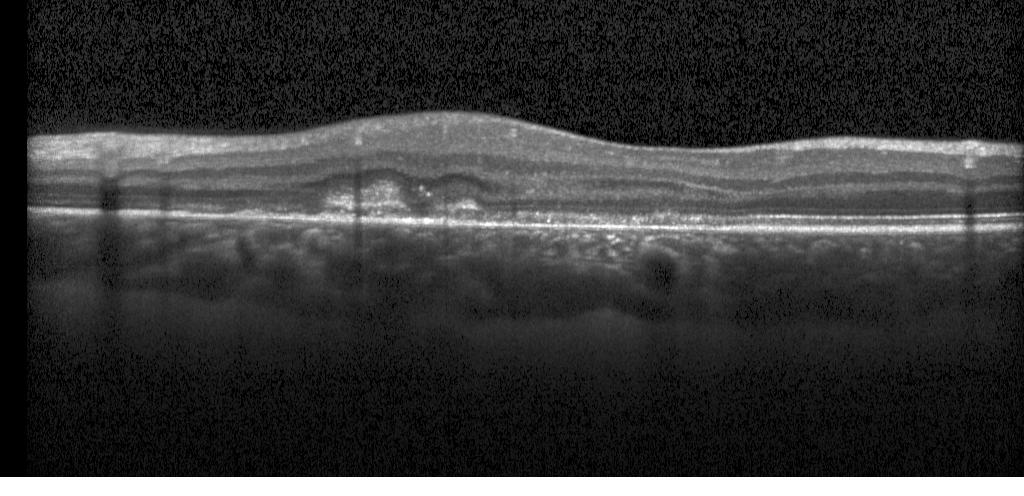

OCT scan showing a choroidal neovascular membrane.